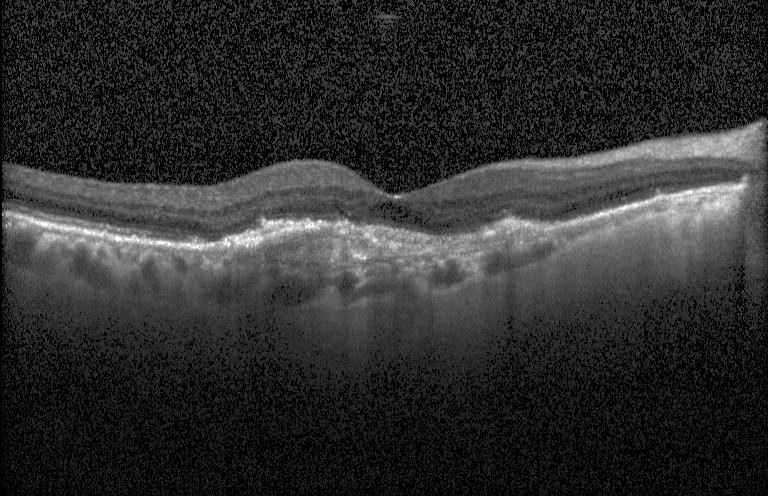 Spectral-domain OCT, retinal OCT B-scan, through the macula.
Finding: choroidal neovascularization.